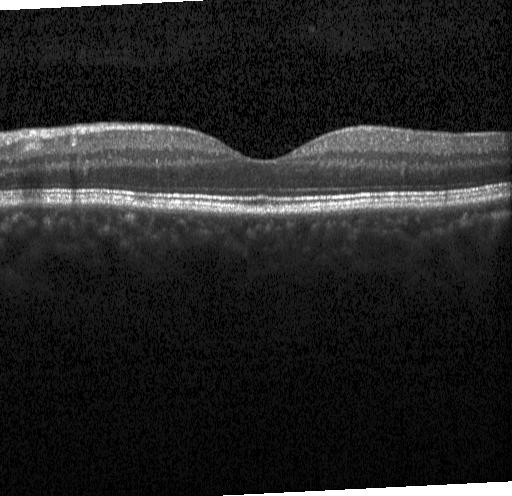

Horizontal scan through the fovea · SD-OCT · OCT line scan. The scan shows no evidence of choroidal neovascularization, diabetic macular edema, or drusen.